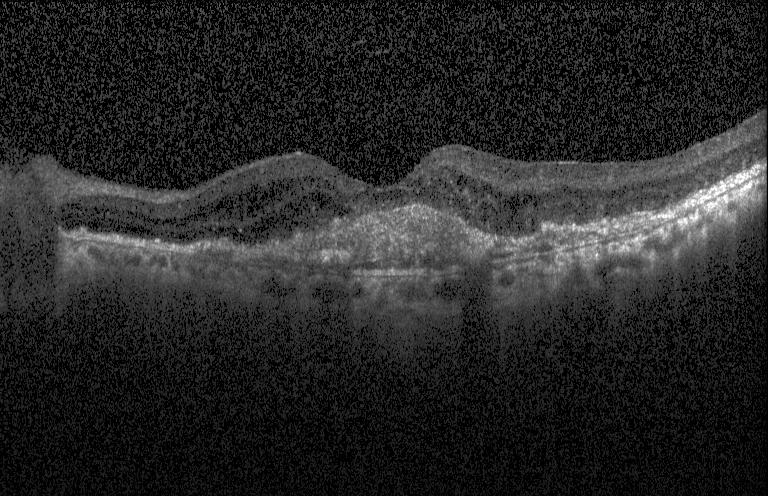 OCT B-scan showing a choroidal neovascular membrane.